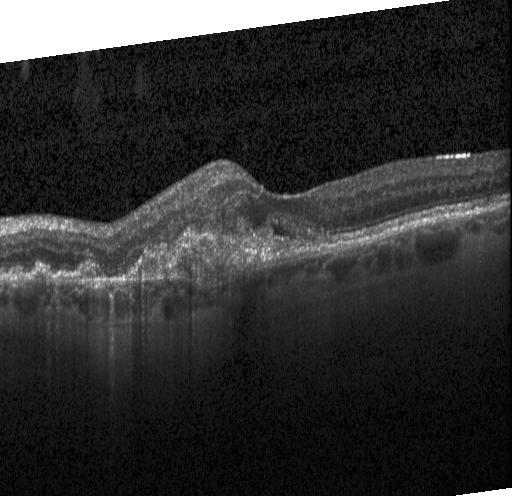 Retinal OCT B-scan. Assessment: a choroidal neovascular membrane.